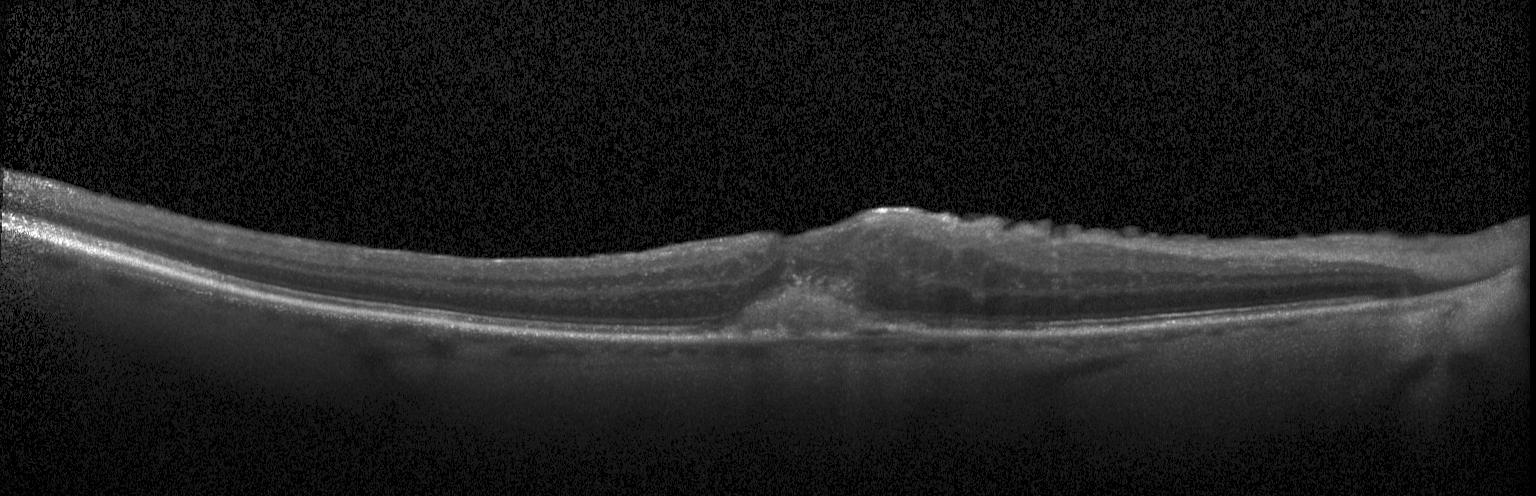
OCT line scan
OCT finding: choroidal neovascularization.